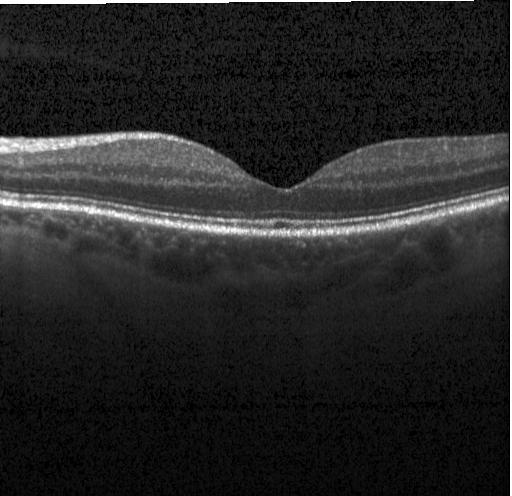 Heidelberg Spectralis OCT system; retinal OCT B-scan — The scan shows no CNV, no DME, and no drusen.